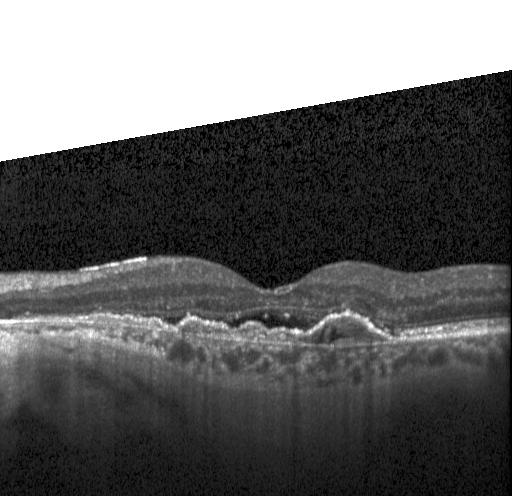
SD-OCT, OCT B-scan, horizontal scan through the fovea
Macular OCT: choroidal neovascularization.